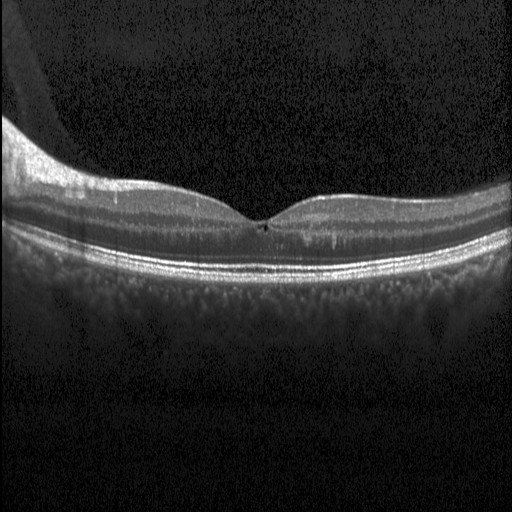 OCT finding: diabetic macular edema.